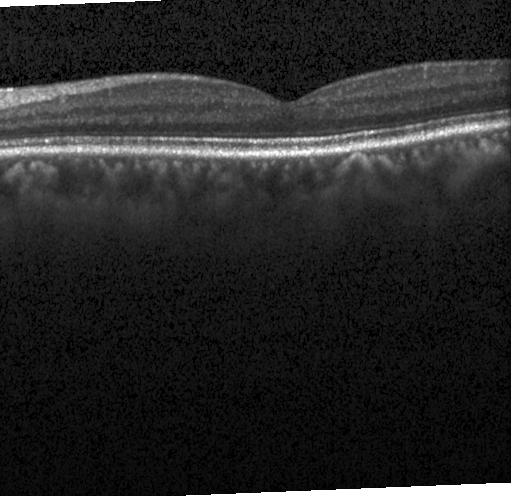
Retinal OCT B-scan. Instrument: Heidelberg Spectralis. Spectral-domain OCT. Fovea-centered. Impression: no choroidal neovascularization, no diabetic macular edema, and no drusen.